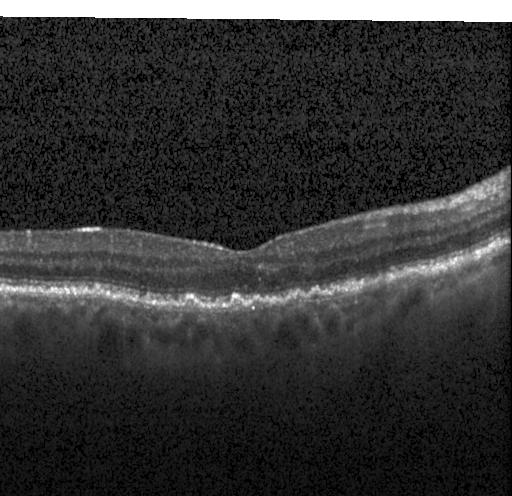 OCT B-scan. Through the macula.
Finding: multiple drusen.